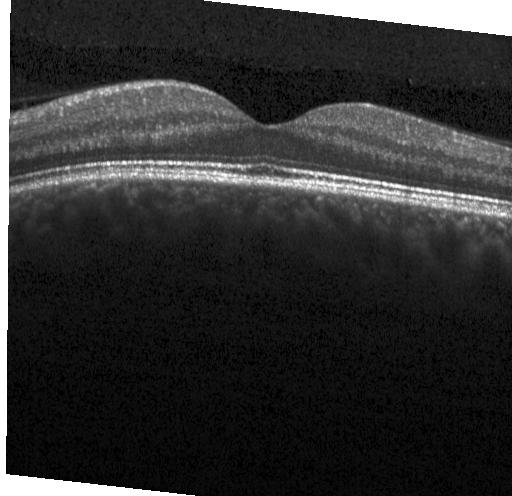

Spectral-domain OCT B-scan: no choroidal neovascularization, diabetic macular edema, or drusen.